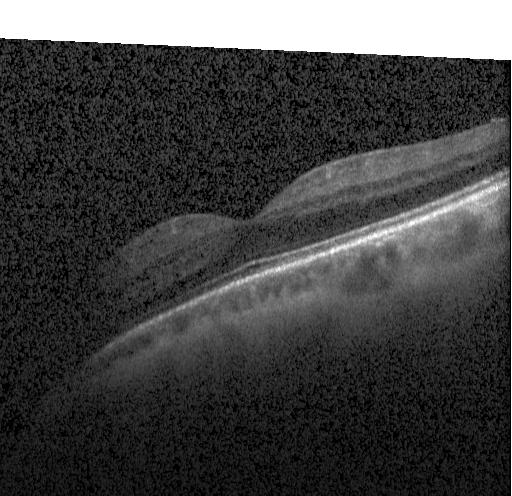 OCT B-scan; acquired on a Heidelberg Spectralis; centered on the fovea; spectral-domain OCT
Neither choroidal neovascularization, diabetic macular edema, nor drusen.